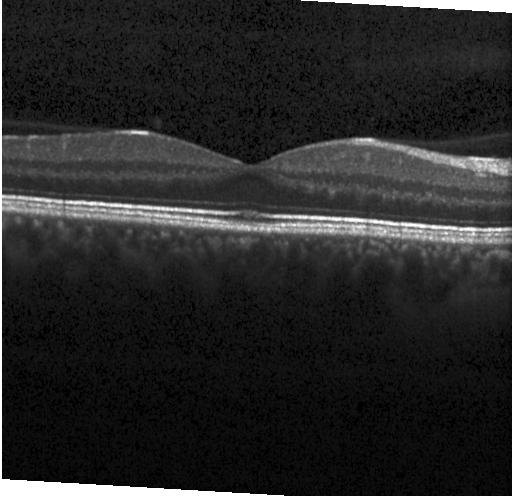
Heidelberg Spectralis OCT system, retinal OCT cross-section, spectral-domain optical coherence tomography, through the macula.
Neither CNV, DME, nor drusen.